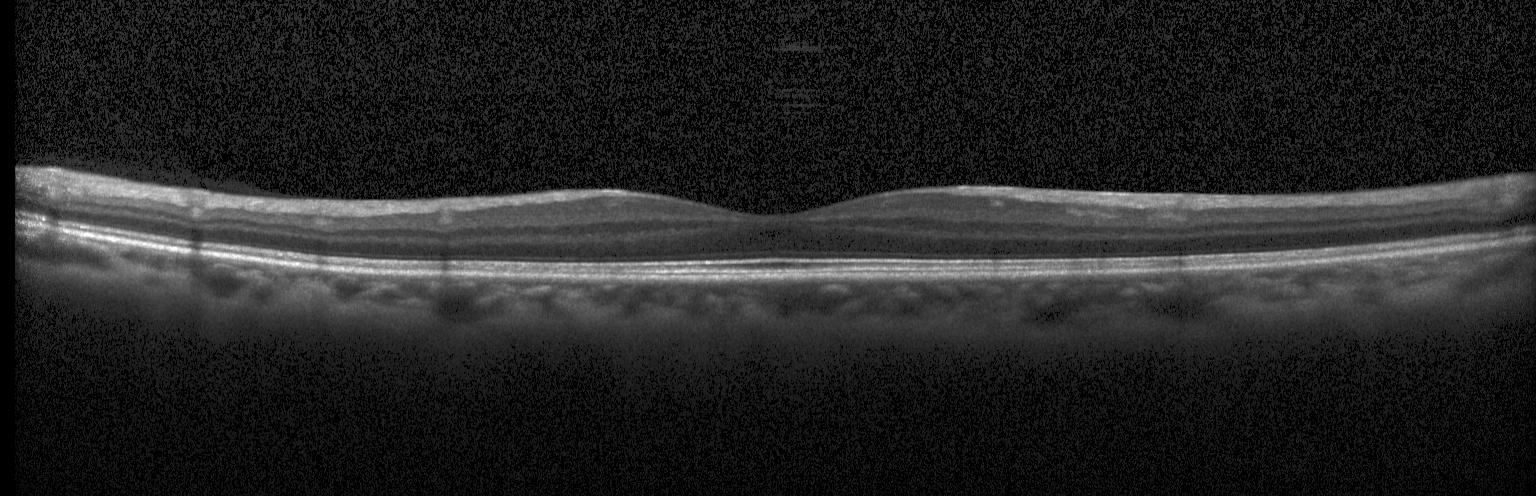 Assessment: no CNV, DME, or drusen.